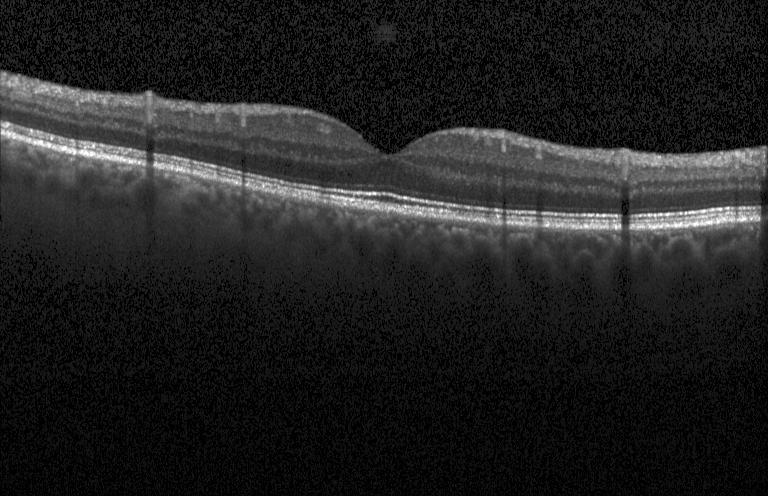 Optical coherence tomography B-scan. Instrument: Heidelberg Spectralis. Horizontal scan through the fovea — Macular OCT: no CNV, DME, or drusen.